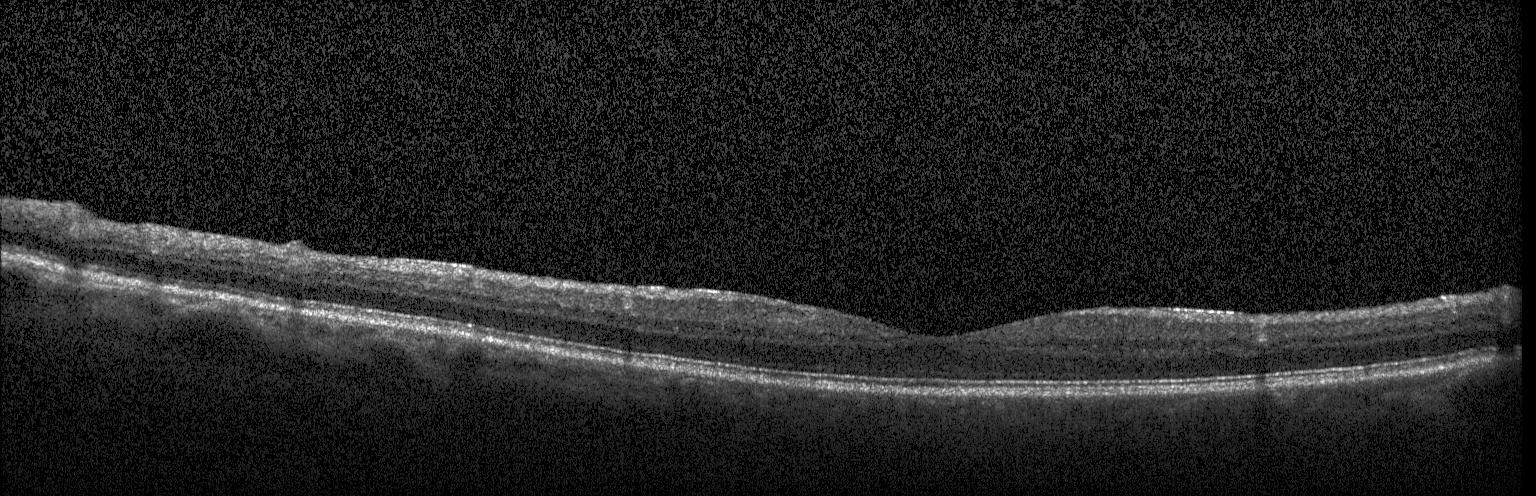 Optical coherence tomography B-scan. Centered on the fovea. Spectral-domain optical coherence tomography — Diagnosis: no CNV, DME, or drusen.